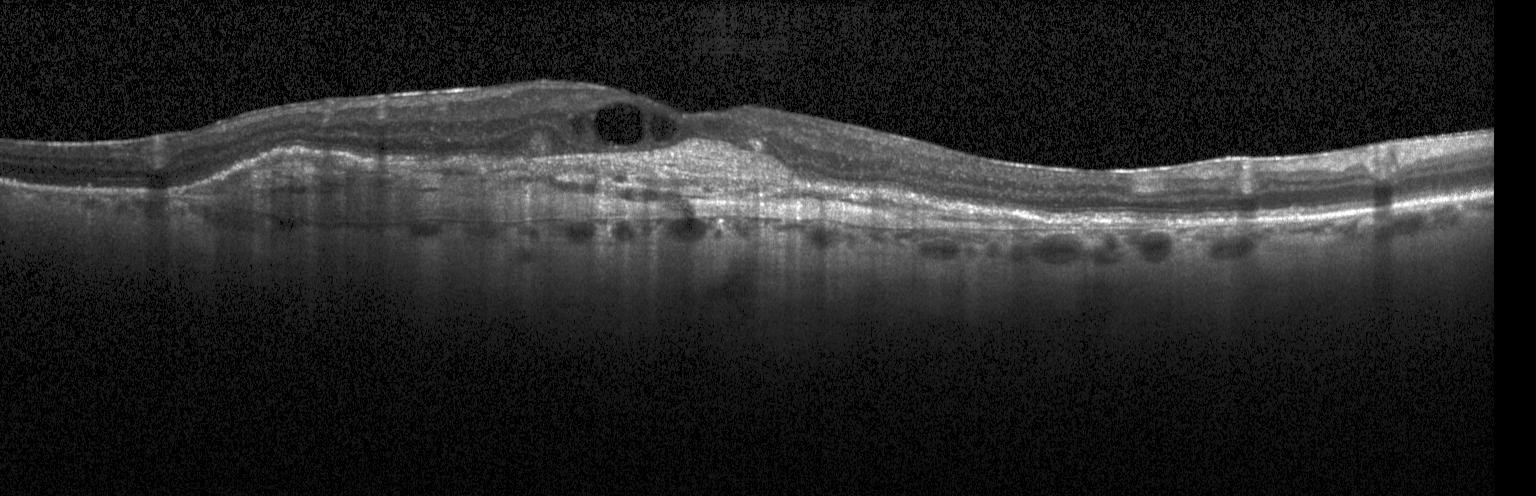

Optical coherence tomography scan, spectral-domain optical coherence tomography
Macular OCT: choroidal neovascularization.